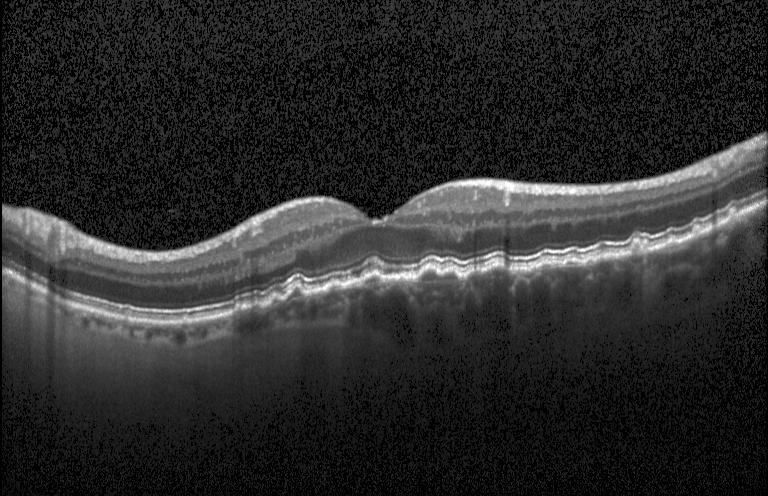
SD-OCT. OCT line scan — Impression: drusen.